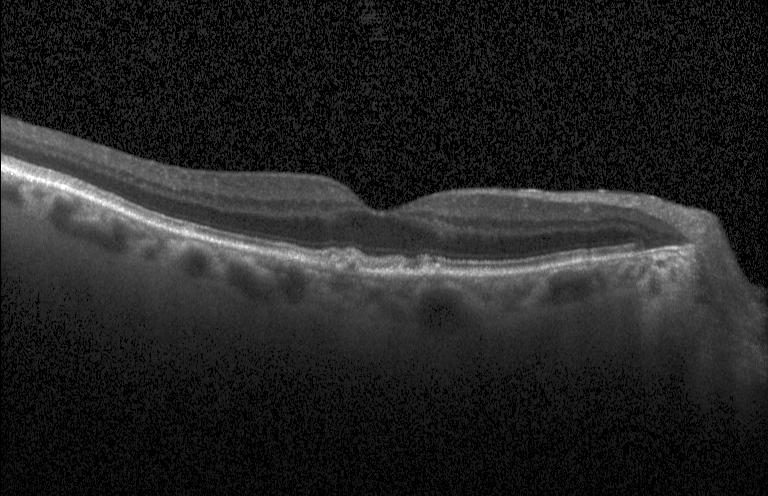 Dx: sub-RPE drusenoid deposits.